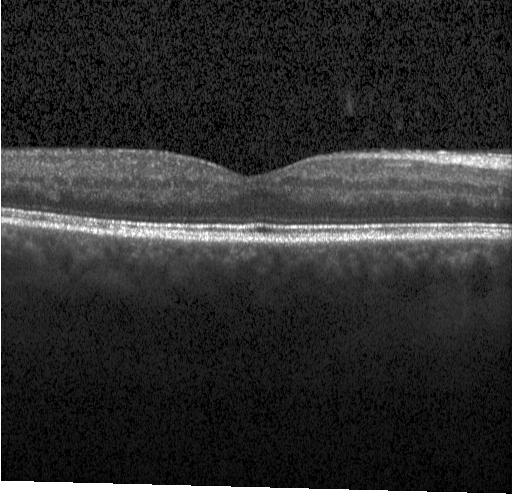 Through the macula · SD-OCT · retinal OCT B-scan · acquired on a Heidelberg Spectralis. Assessment: no CNV, DME, or drusen.